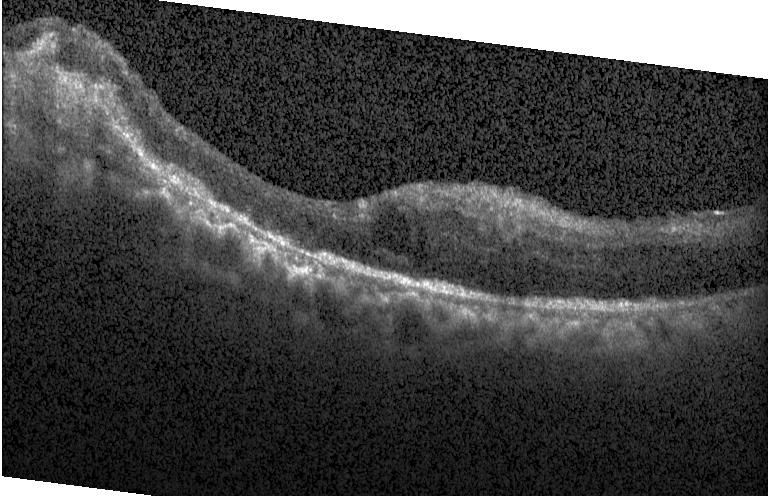
Retinal OCT B-scan. Fovea-centered
Finding: a choroidal neovascular membrane.